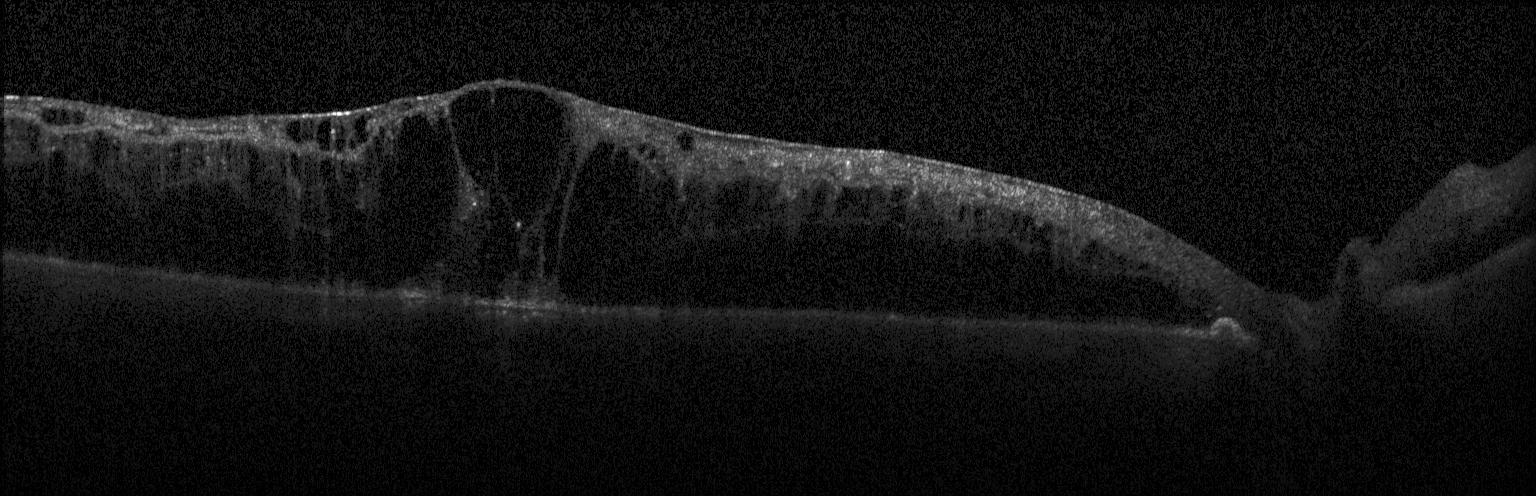

SD-OCT, Heidelberg Spectralis, optical coherence tomography B-scan
This B-scan demonstrates diabetic macular edema.